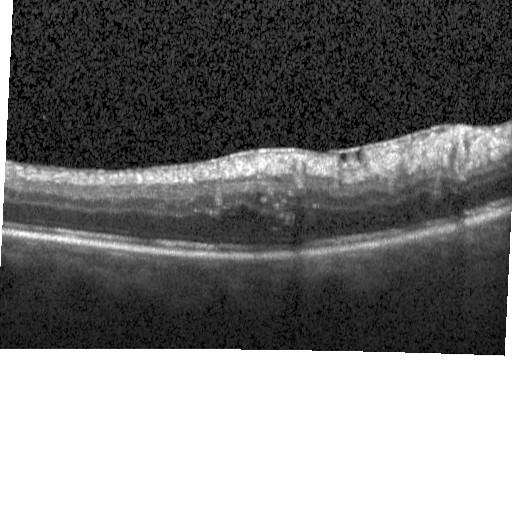
OCT finding: diabetic macular edema.